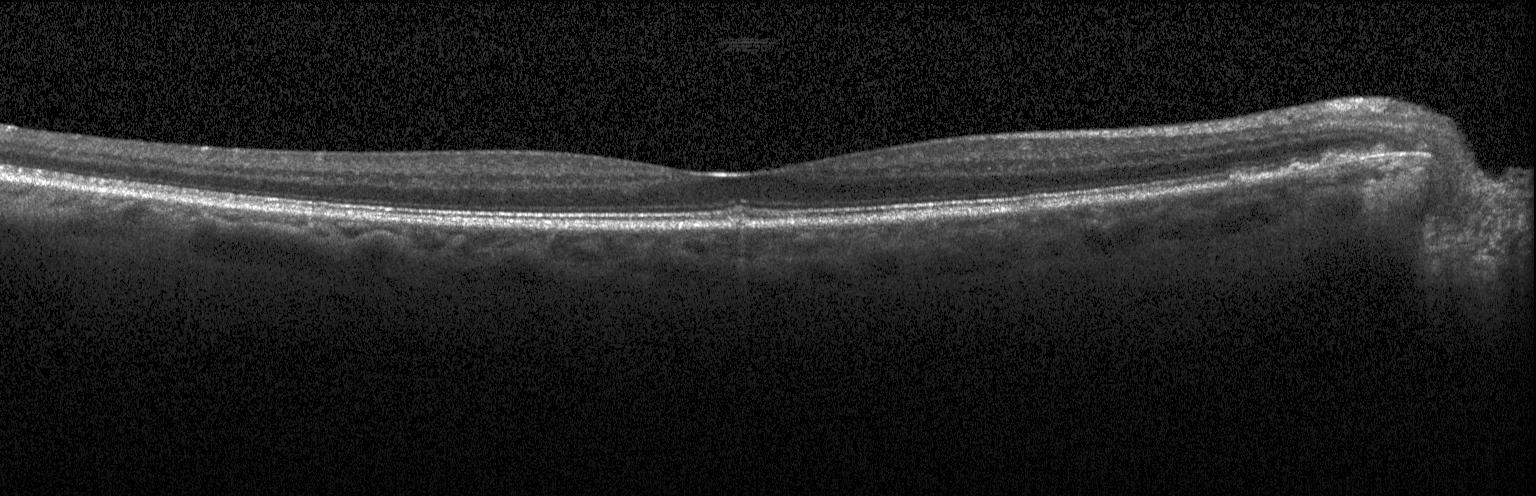
Impression: no choroidal neovascularization, diabetic macular edema, or drusen.